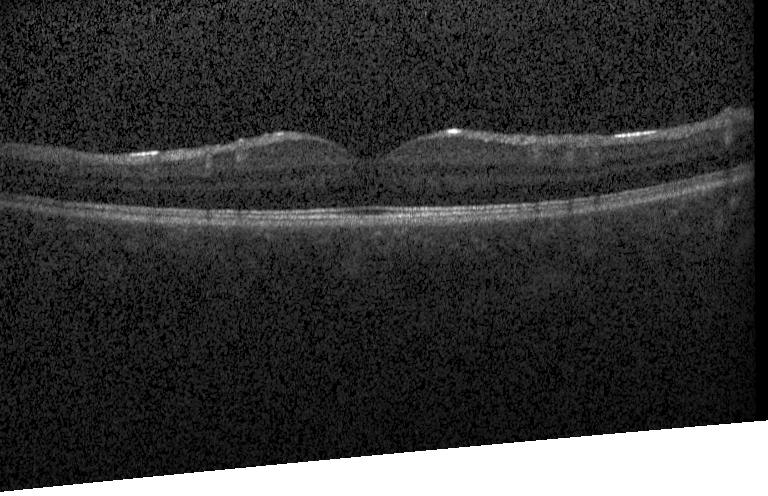 Acquired on a Heidelberg Spectralis · fovea-centered · retinal OCT cross-section.
This B-scan demonstrates no choroidal neovascularization, diabetic macular edema, or drusen.